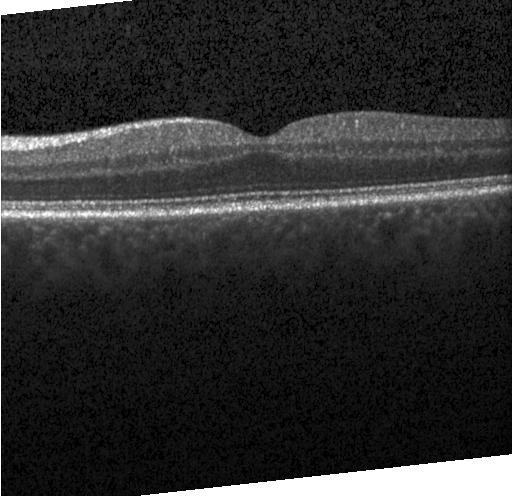
Spectral-domain optical coherence tomography, centered on the fovea, Heidelberg Spectralis OCT system, retinal OCT cross-section — Finding: no choroidal neovascularization, no diabetic macular edema, and no drusen.